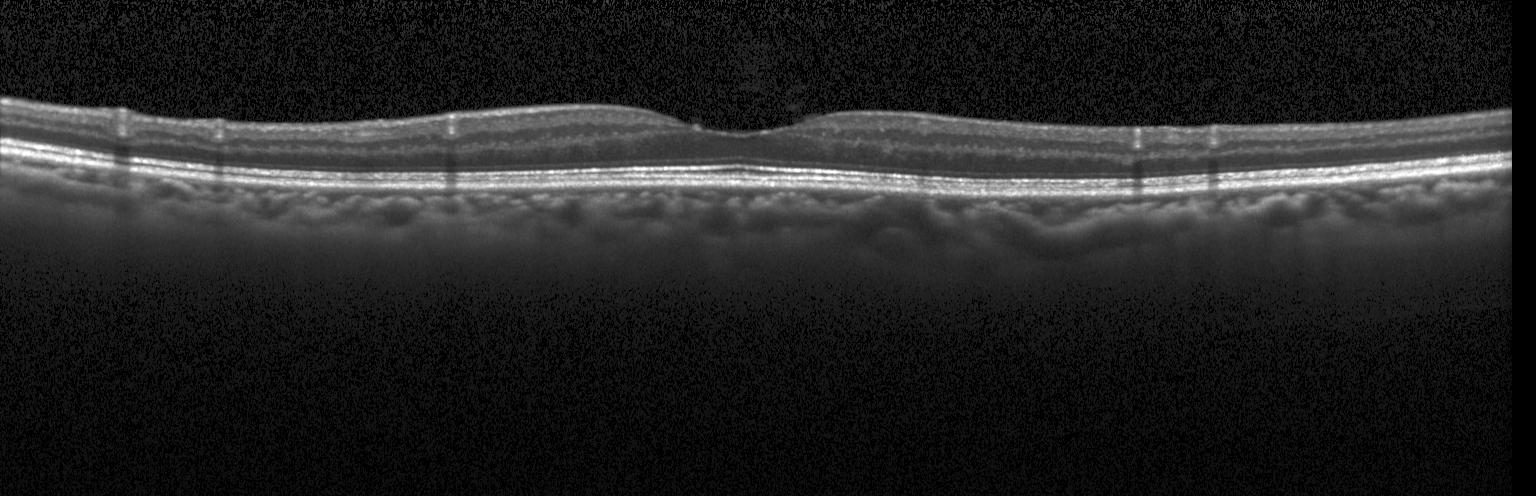

OCT scan showing no CNV, DME, or drusen.